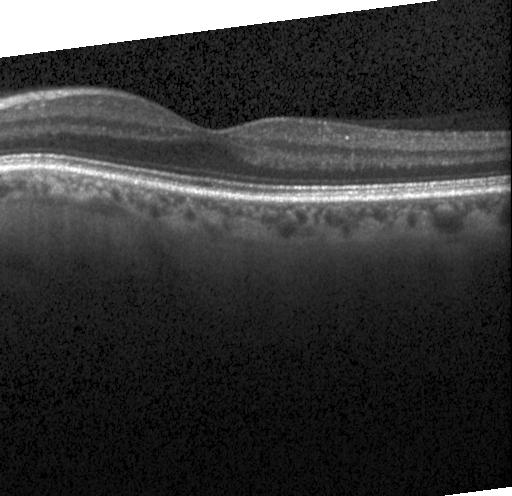 Assessment: no choroidal neovascularization, diabetic macular edema, or drusen.